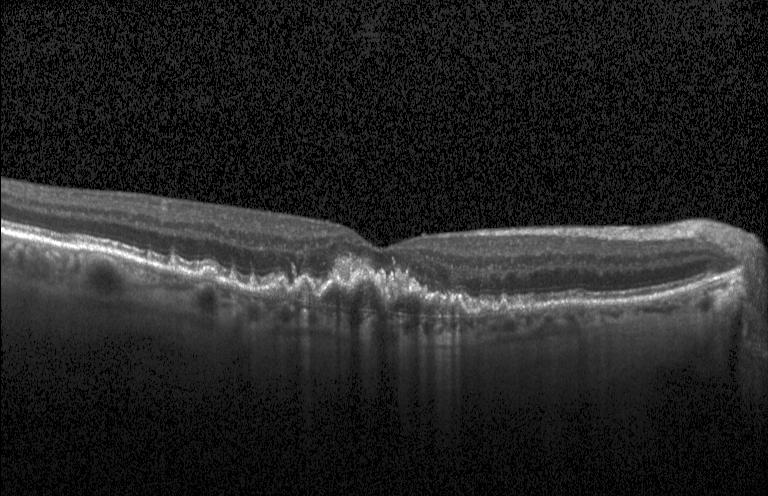
Assessment: a choroidal neovascular membrane.